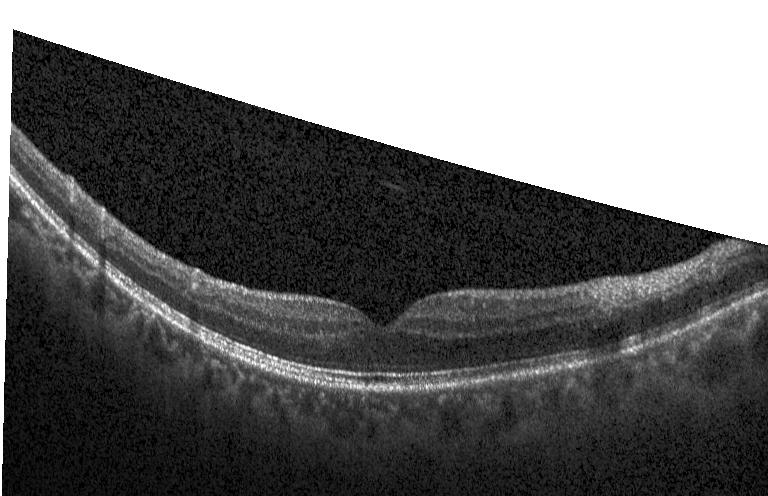

Impression: no CNV, no DME, and no drusen.